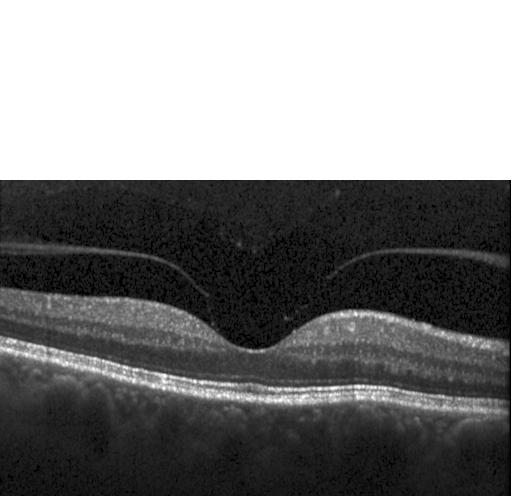
Horizontal scan through the fovea, retinal OCT B-scan.
Finding: neither CNV, DME, nor drusen.